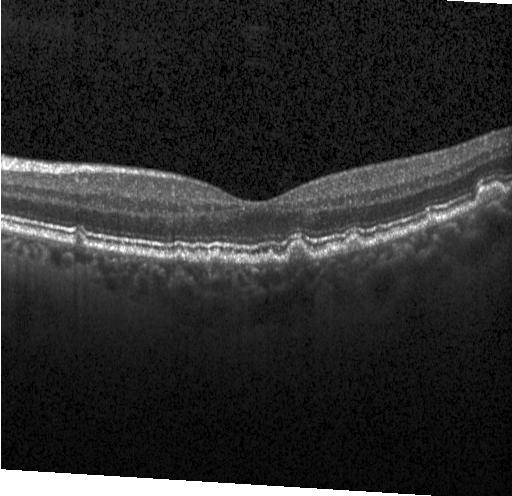

Diagnosis: drusen.